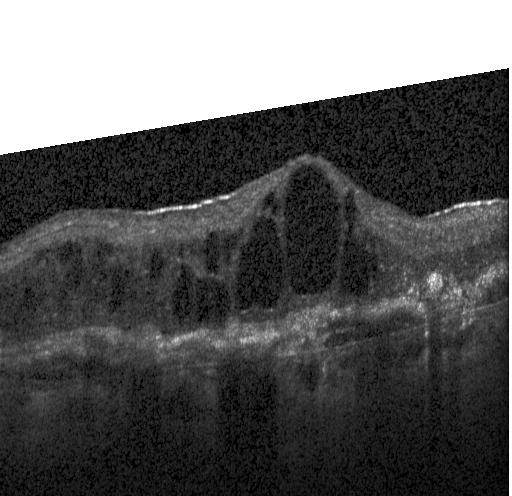
Heidelberg Spectralis; retinal OCT B-scan; centered on the fovea — Impression: a choroidal neovascular membrane.